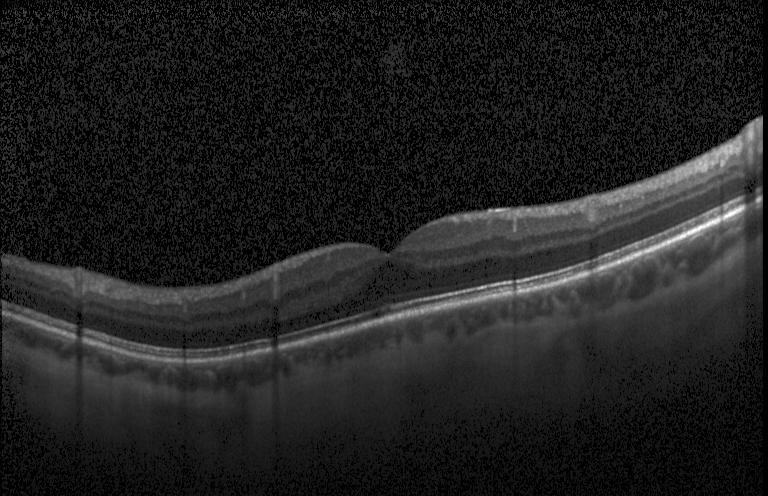 OCT line scan — Neither CNV, DME, nor drusen.